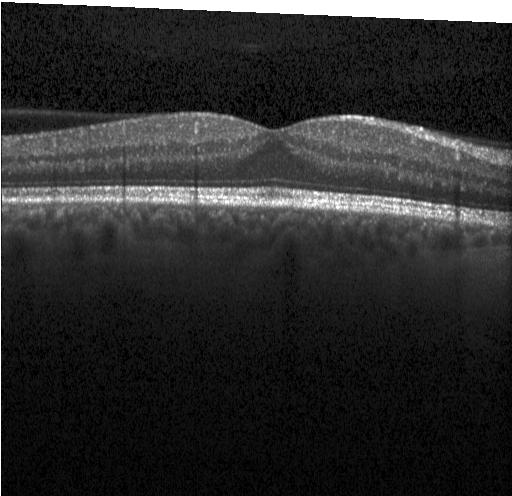
SD-OCT; OCT line scan; horizontal scan through the fovea. This B-scan demonstrates no choroidal neovascularization, no diabetic macular edema, and no drusen.